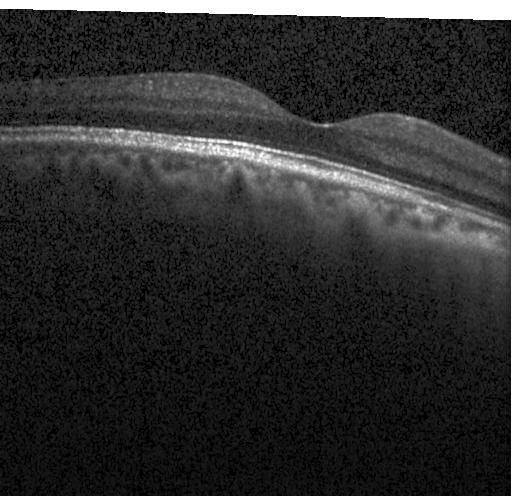
OCT scan showing no evidence of choroidal neovascularization, diabetic macular edema, or drusen.